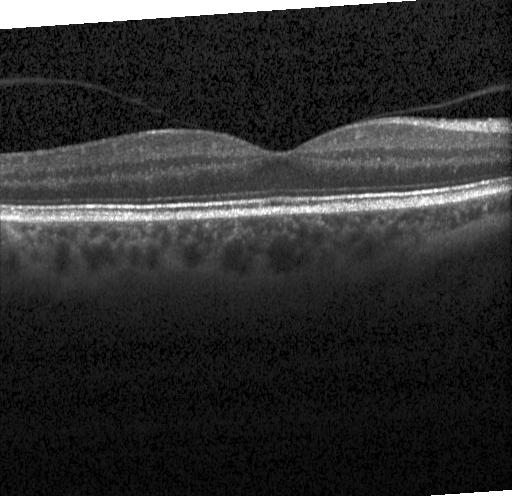
Diagnosis: no choroidal neovascularization, no diabetic macular edema, and no drusen.